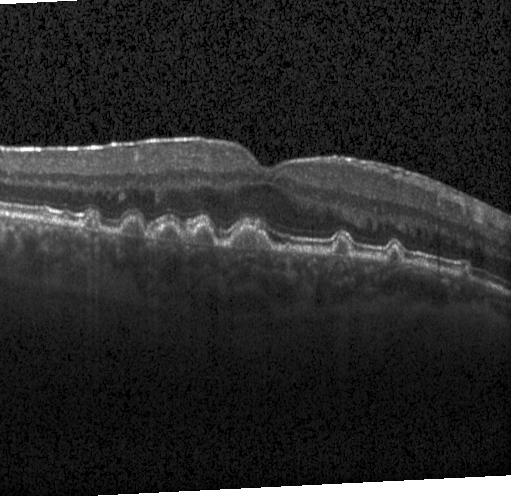 Impression: multiple drusen.